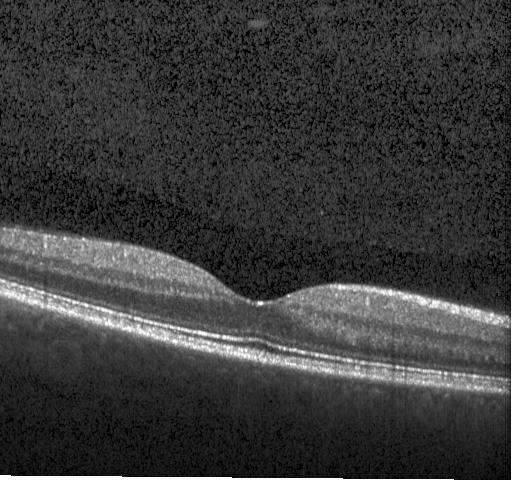 Retinal OCT cross-section. Impression: no evidence of choroidal neovascularization, diabetic macular edema, or drusen.